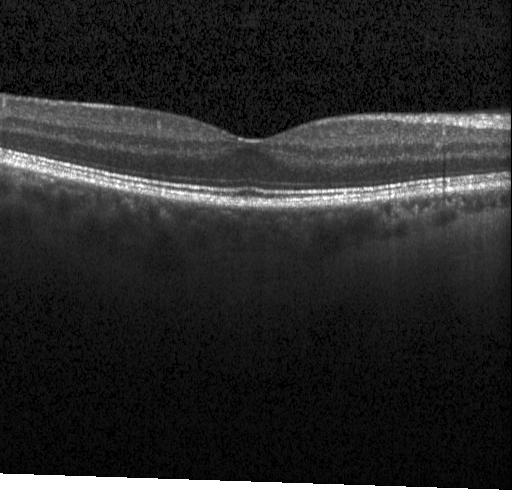

Macular OCT demonstrating no evidence of CNV, DME, or drusen.